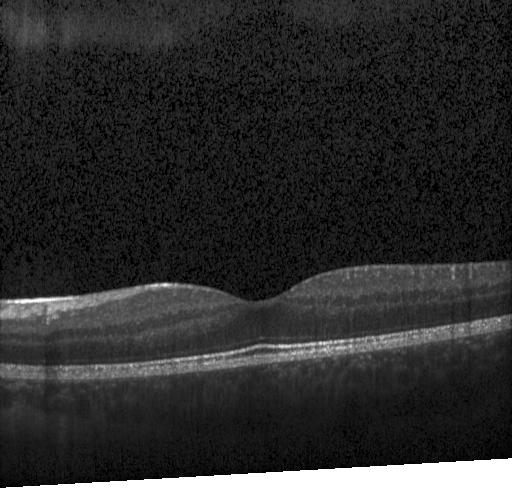 Dx: neither choroidal neovascularization, diabetic macular edema, nor drusen.